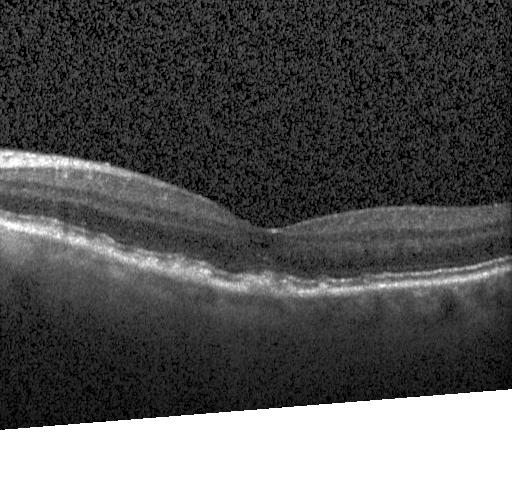
Optical coherence tomography scan
Diagnosis: sub-RPE drusenoid deposits.